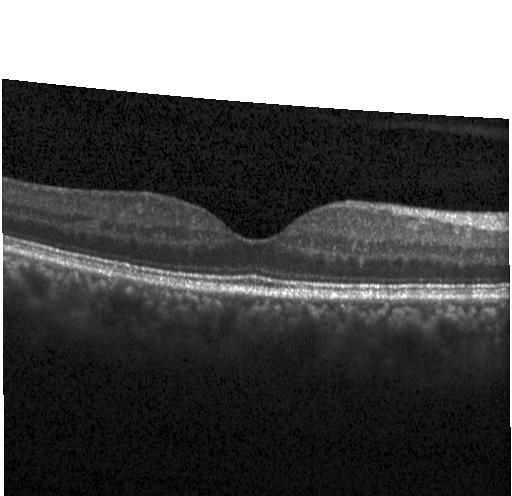
Impression: no CNV, no DME, and no drusen.